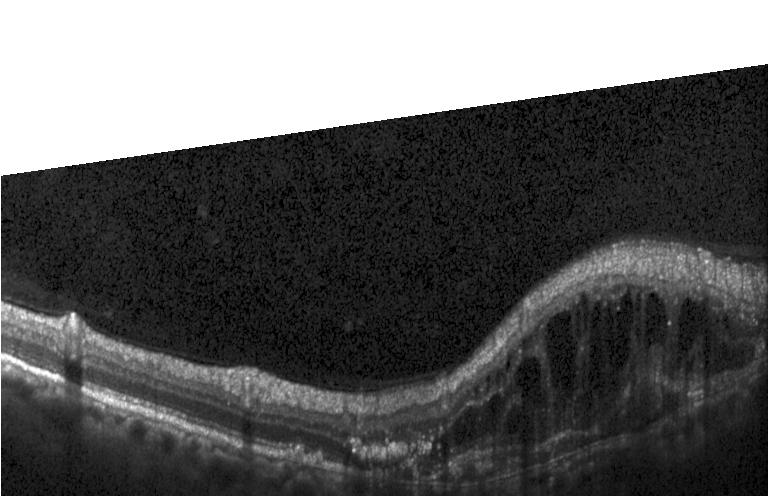 Assessment: CNV.